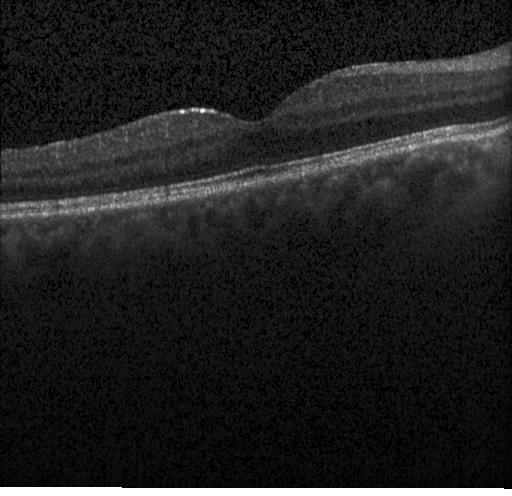 Spectral-domain OCT · acquired on a Heidelberg Spectralis · retinal OCT cross-section · fovea-centered. Diagnosis: neither choroidal neovascularization, diabetic macular edema, nor drusen.